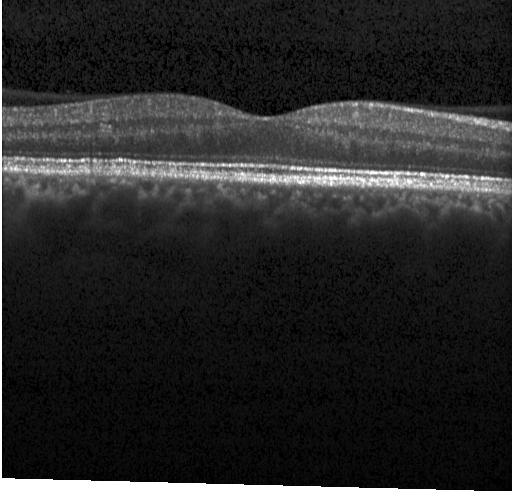 OCT line scan. Dx: neither choroidal neovascularization, diabetic macular edema, nor drusen.